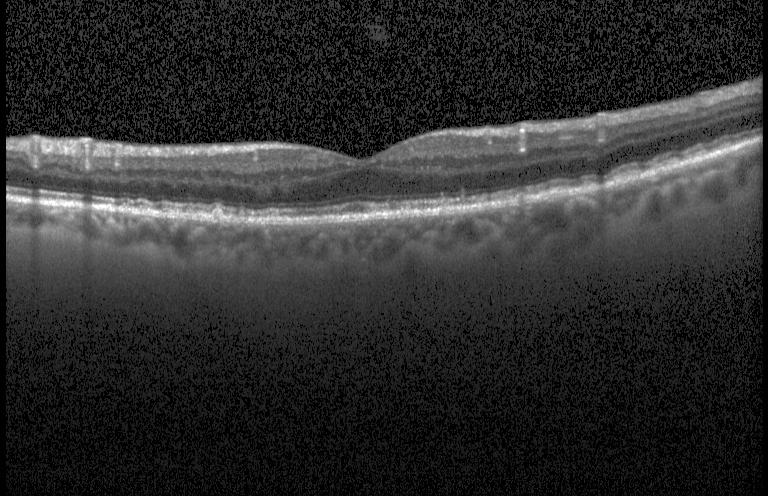 Horizontal scan through the fovea · Heidelberg Spectralis OCT system · optical coherence tomography scan · spectral-domain optical coherence tomography.
Finding: sub-RPE drusenoid deposits.